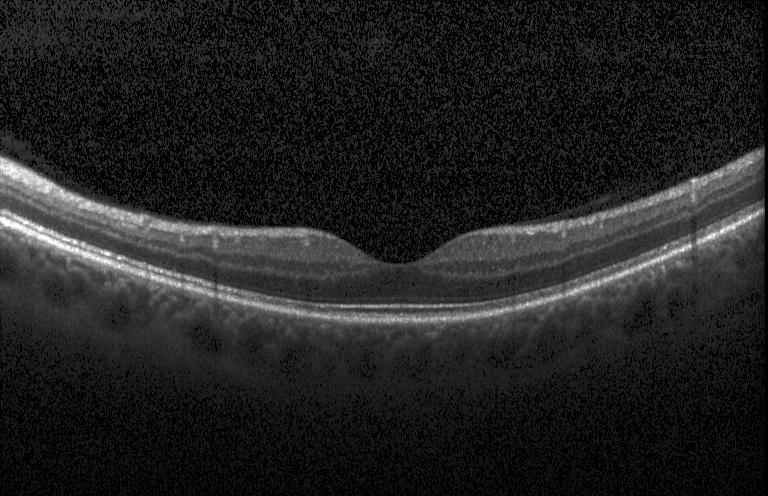
Retinal OCT cross-section · spectral-domain optical coherence tomography.
Diagnosis: neither CNV, DME, nor drusen.